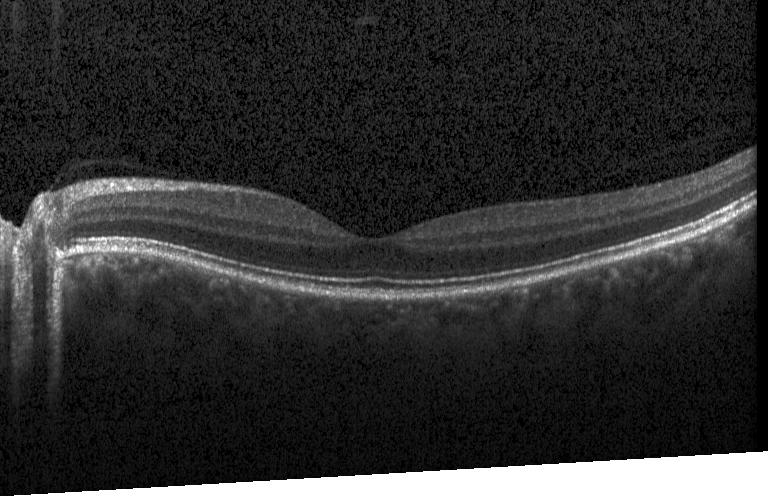

Diagnosis: neither CNV, DME, nor drusen.